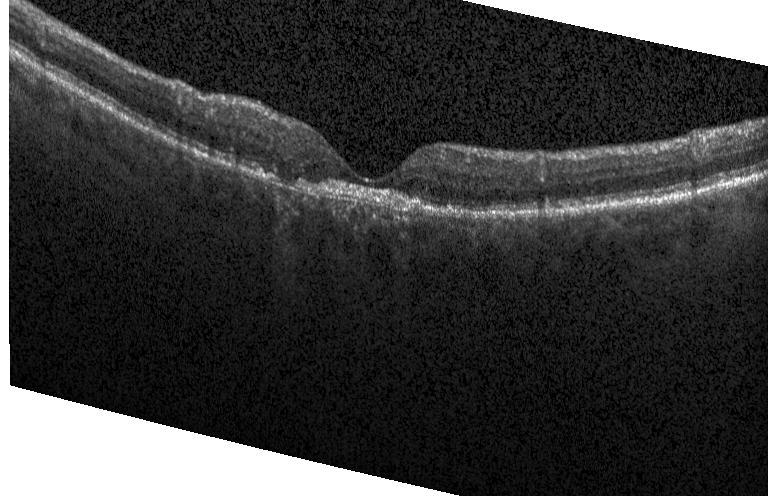

Impression: choroidal neovascularization.